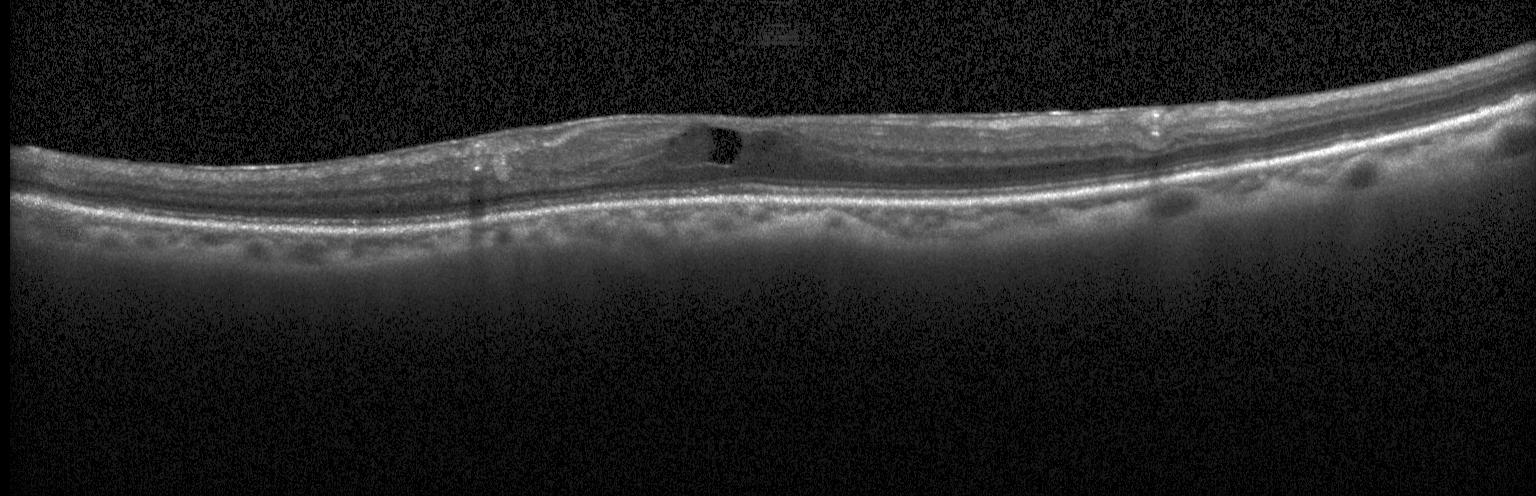 Dx: DME.